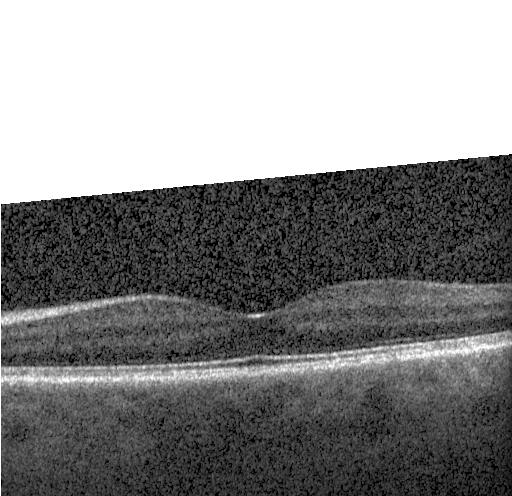
Fovea-centered · spectral-domain OCT · retinal OCT B-scan.
Dx: no evidence of choroidal neovascularization, diabetic macular edema, or drusen.